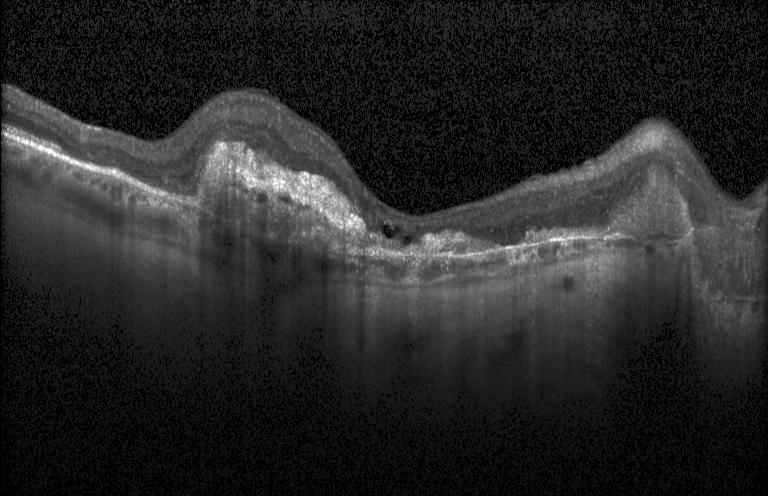

Macular OCT: CNV.